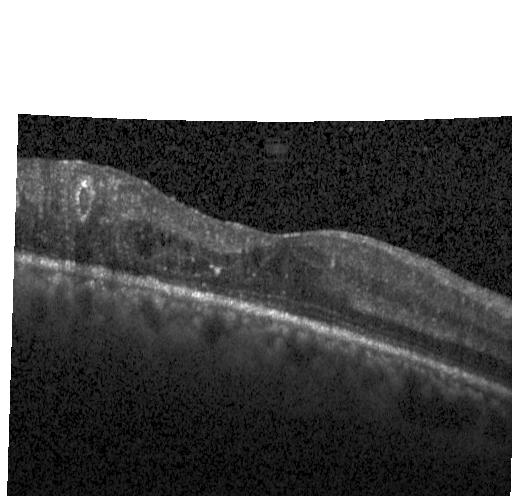 Optical coherence tomography B-scan; spectral-domain optical coherence tomography; horizontal scan through the fovea; acquired on a Heidelberg Spectralis
Finding: diabetic macular edema (DME).